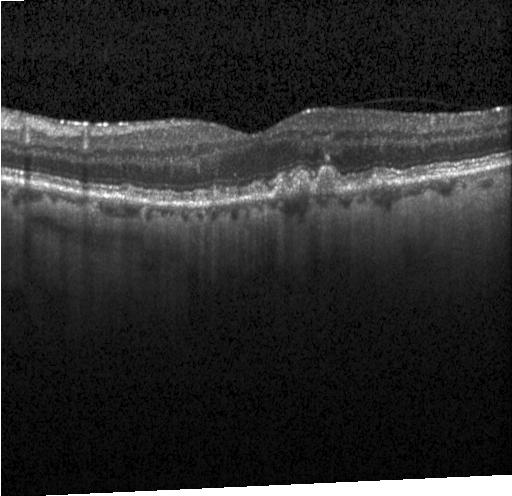 Retinal OCT cross-section. Instrument: Heidelberg Spectralis. Spectral-domain OCT. Assessment: sub-RPE drusenoid deposits.